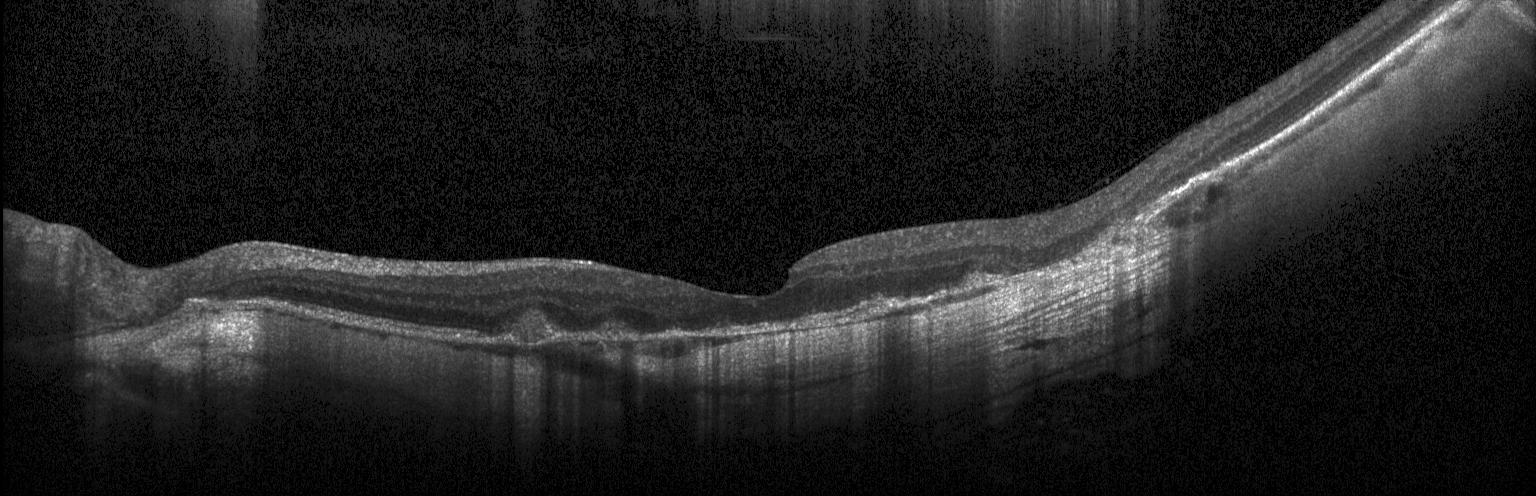

Impression: CNV.